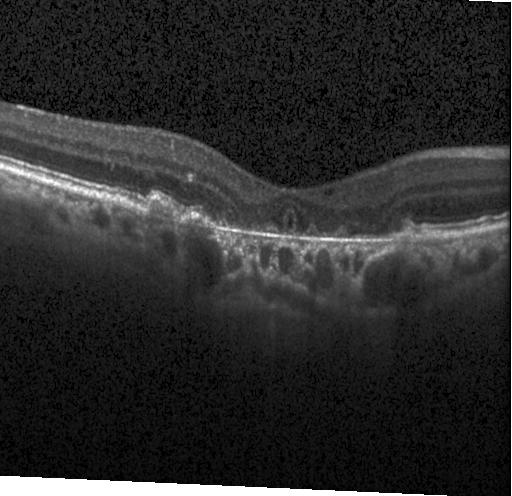 OCT line scan — Assessment: a choroidal neovascular membrane.